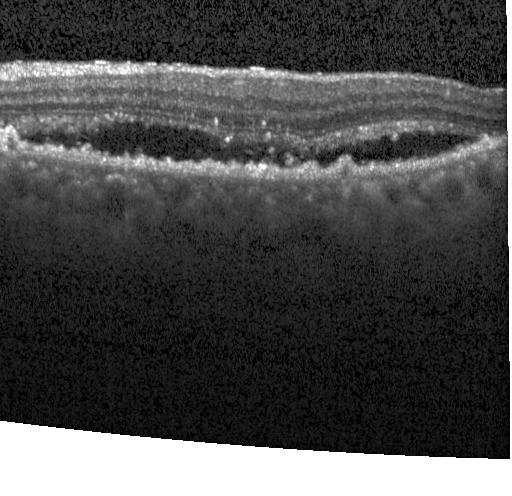

Retinal OCT B-scan; acquired on a Heidelberg Spectralis
Assessment: CNV.